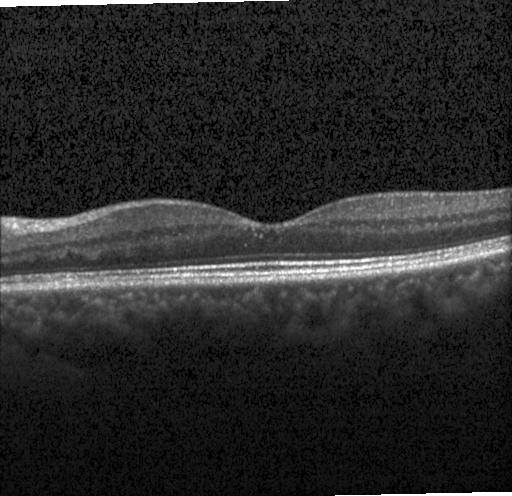 OCT B-scan — Dx: no choroidal neovascularization, diabetic macular edema, or drusen.